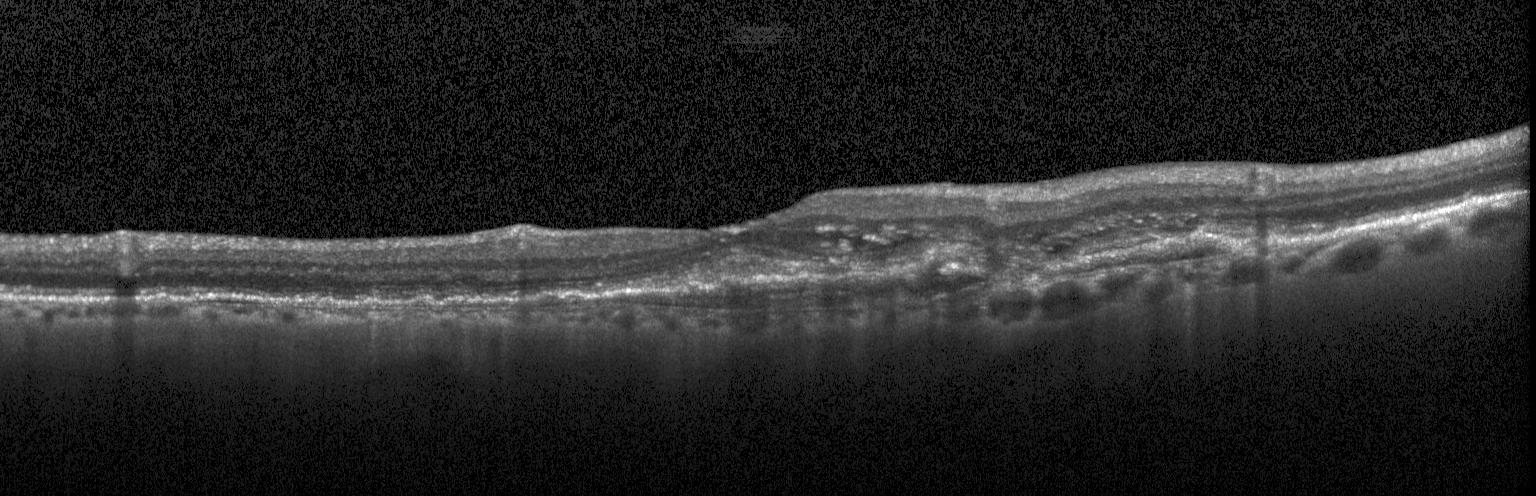 Impression: choroidal neovascularization.